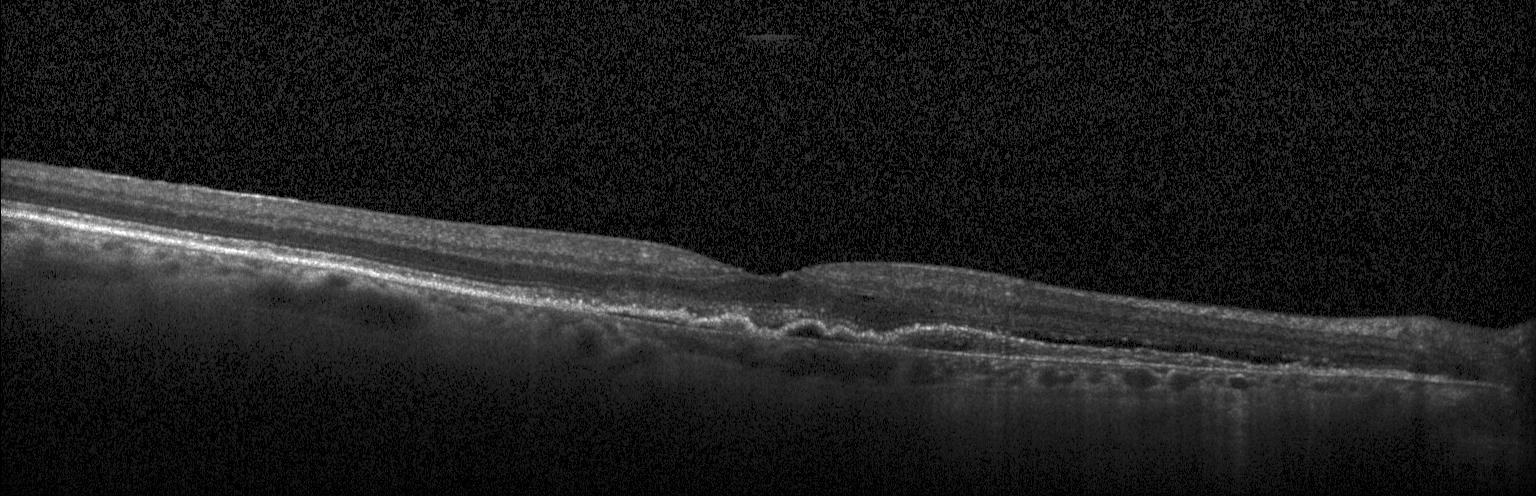

Macular scan, acquired on a Heidelberg Spectralis, retinal OCT B-scan, spectral-domain OCT.
Diagnosis: a choroidal neovascular membrane.